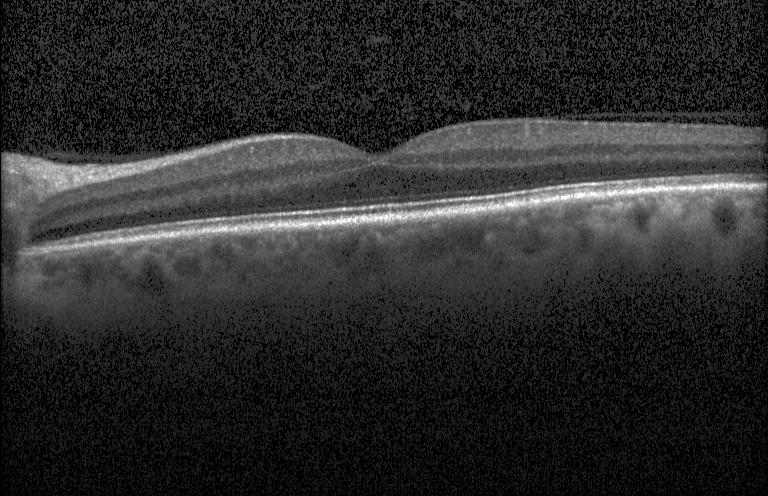

Assessment: neither CNV, DME, nor drusen.